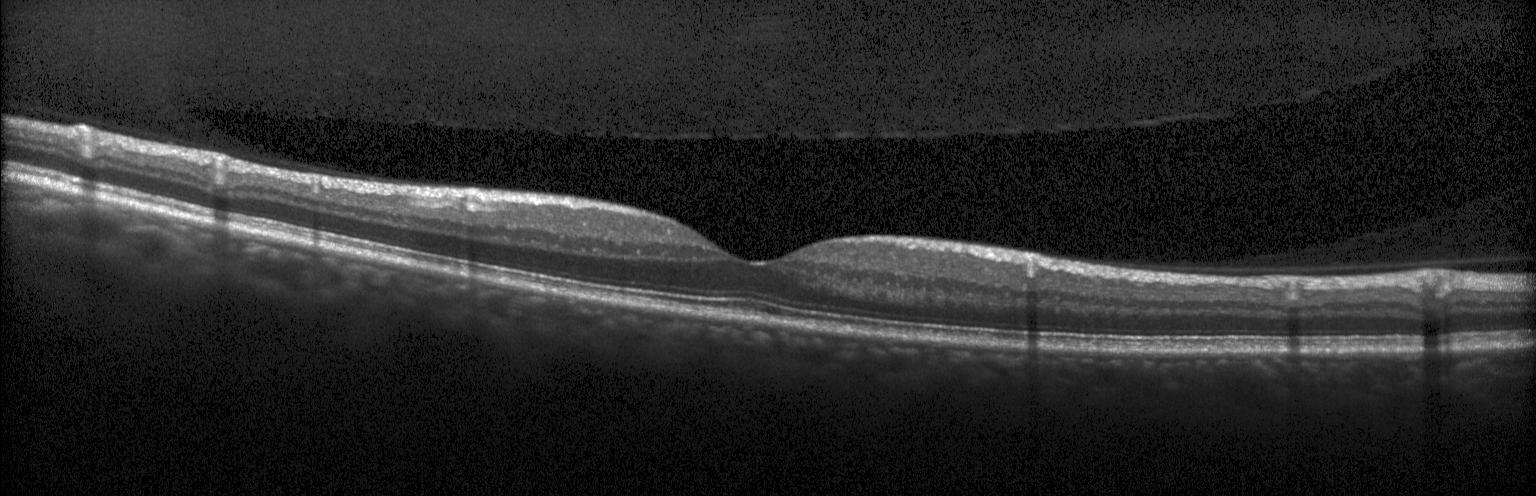
Heidelberg Spectralis. Retinal OCT cross-section. Spectral-domain OCT
Impression: neither CNV, DME, nor drusen.